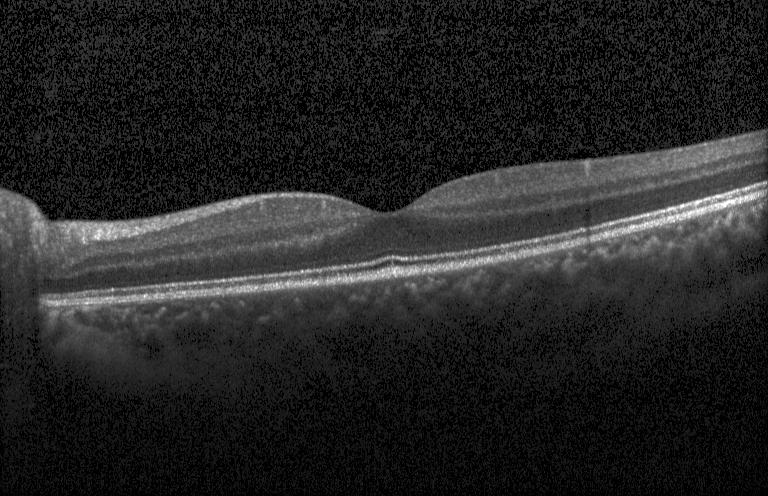

Heidelberg Spectralis; OCT line scan; SD-OCT; horizontal scan through the fovea
Assessment: neither CNV, DME, nor drusen.